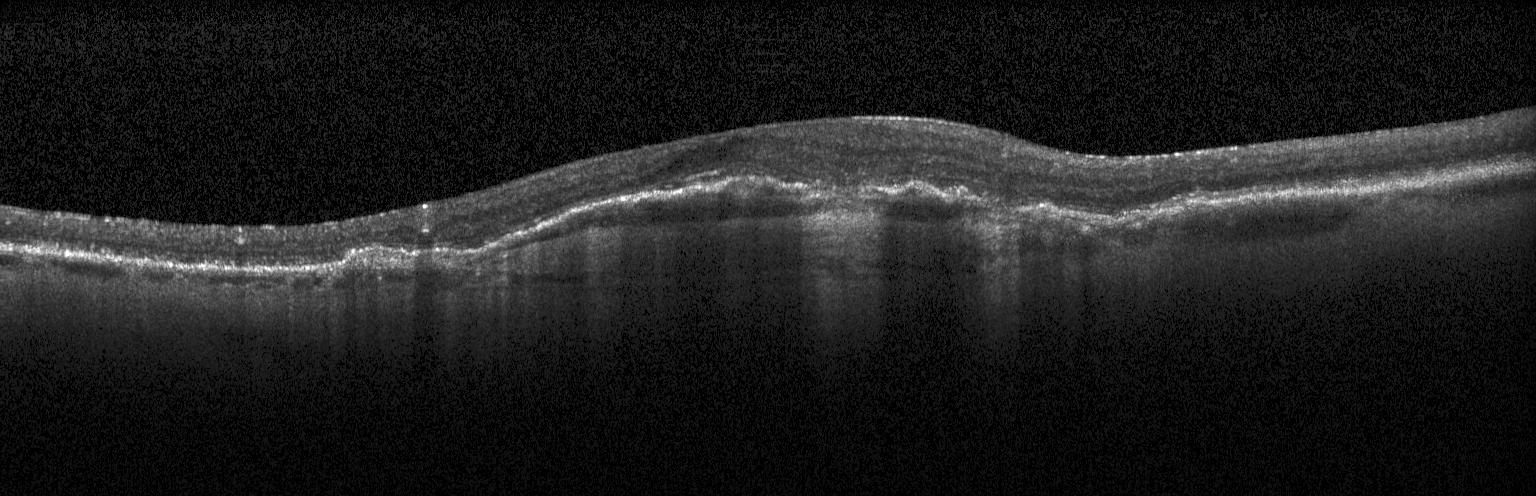
OCT B-scan
Diagnosis: choroidal neovascularization.